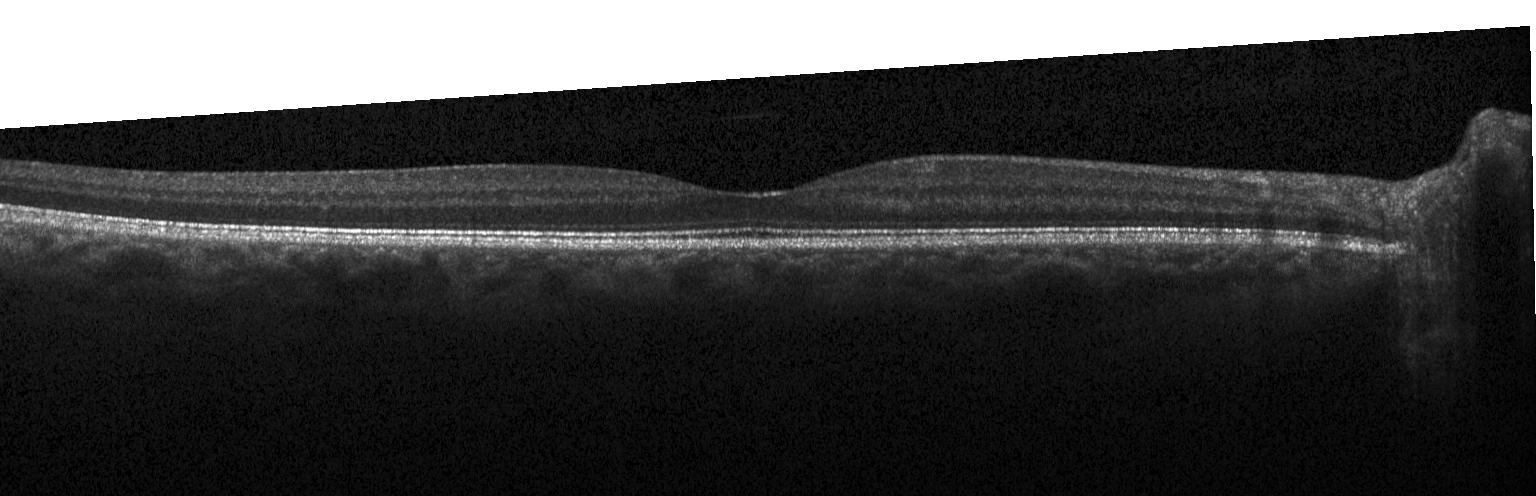 Instrument: Heidelberg Spectralis · retinal OCT cross-section · macular scan
Assessment: neither CNV, DME, nor drusen.